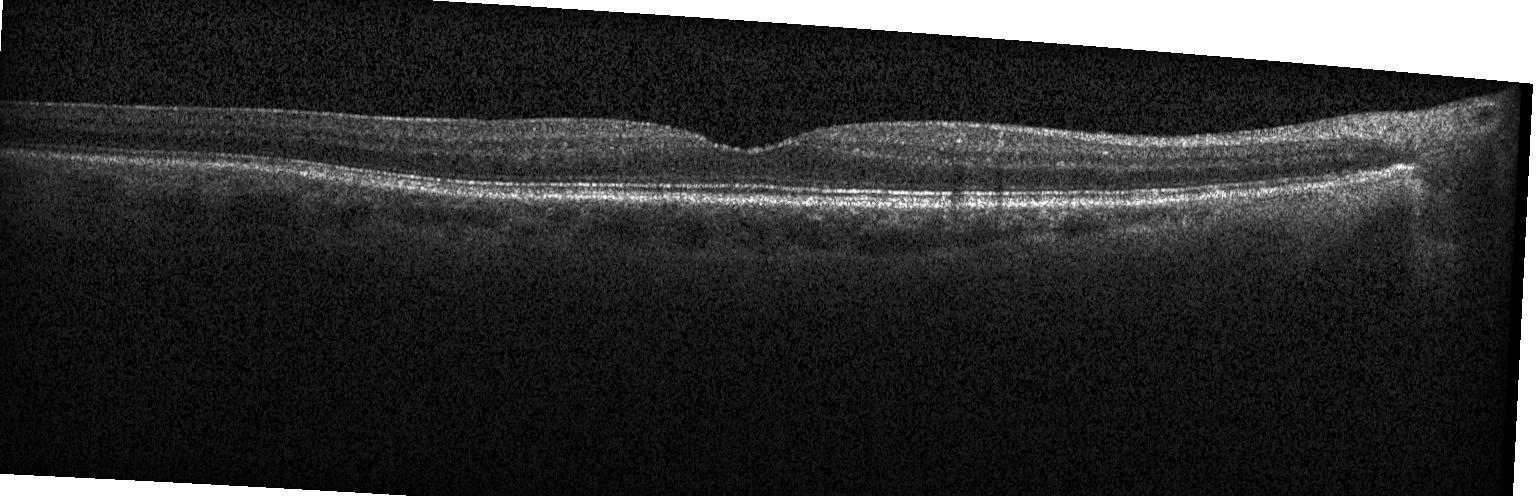
Optical coherence tomography scan — Impression: neither CNV, DME, nor drusen.